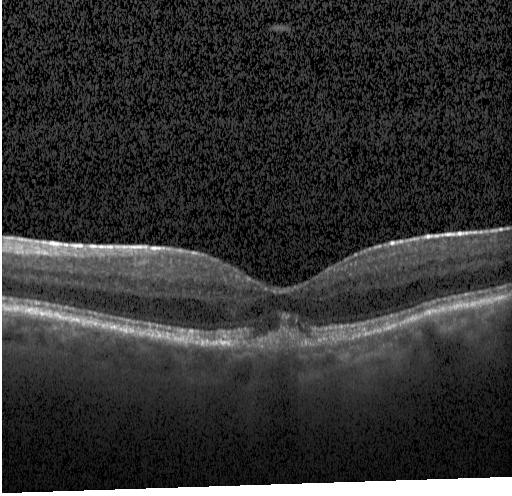
Optical coherence tomography scan · spectral-domain optical coherence tomography · Heidelberg Spectralis OCT system. The scan shows choroidal neovascularization (CNV).